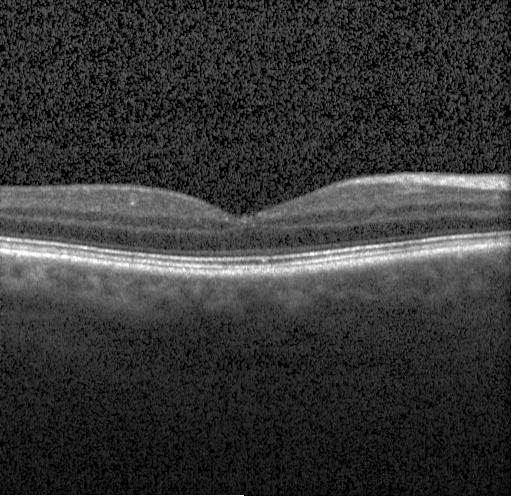
Retinal OCT B-scan. Spectral-domain OCT. OCT finding: no evidence of choroidal neovascularization, diabetic macular edema, or drusen.